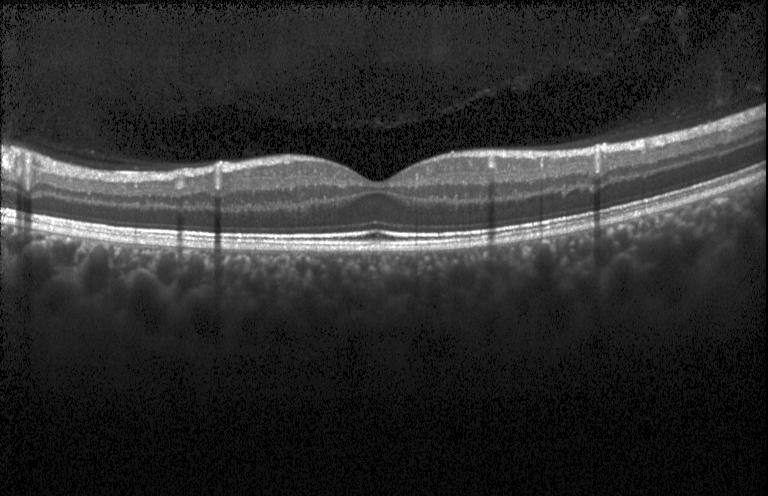
Diagnosis: no evidence of choroidal neovascularization, diabetic macular edema, or drusen.